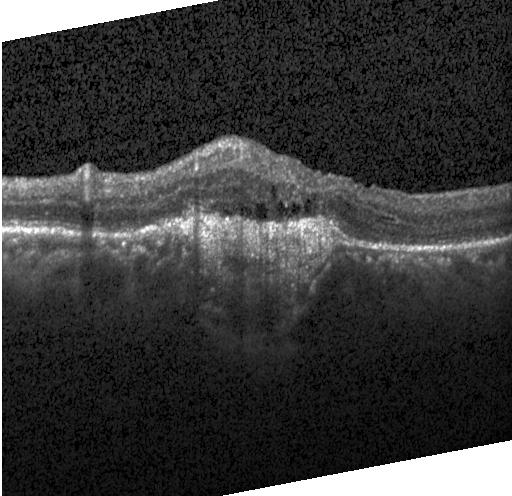 OCT scan showing CNV.